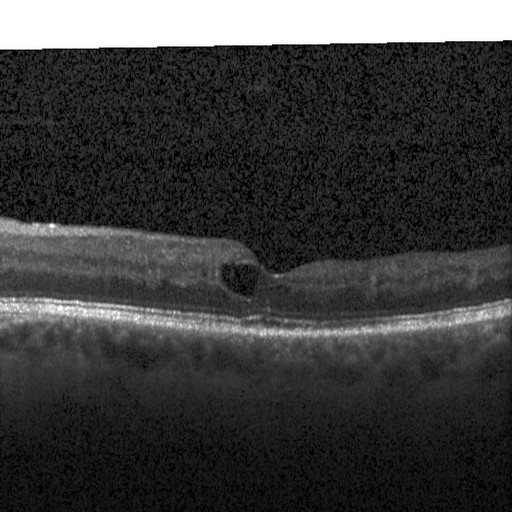 Diagnosis: DME.